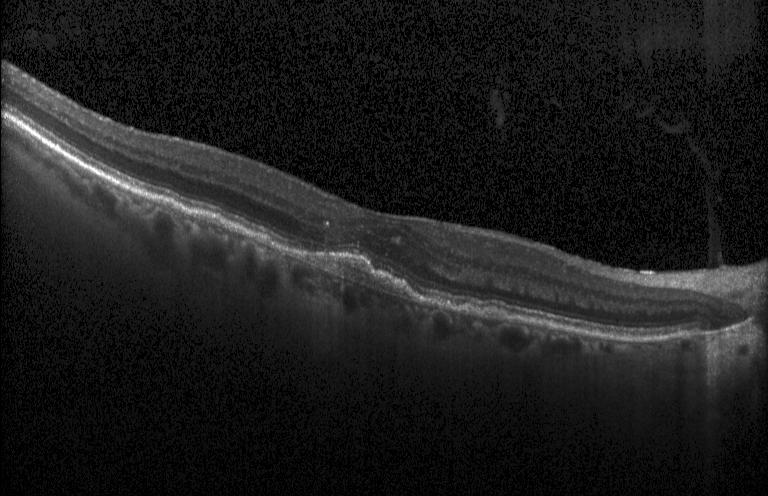
OCT finding: CNV.